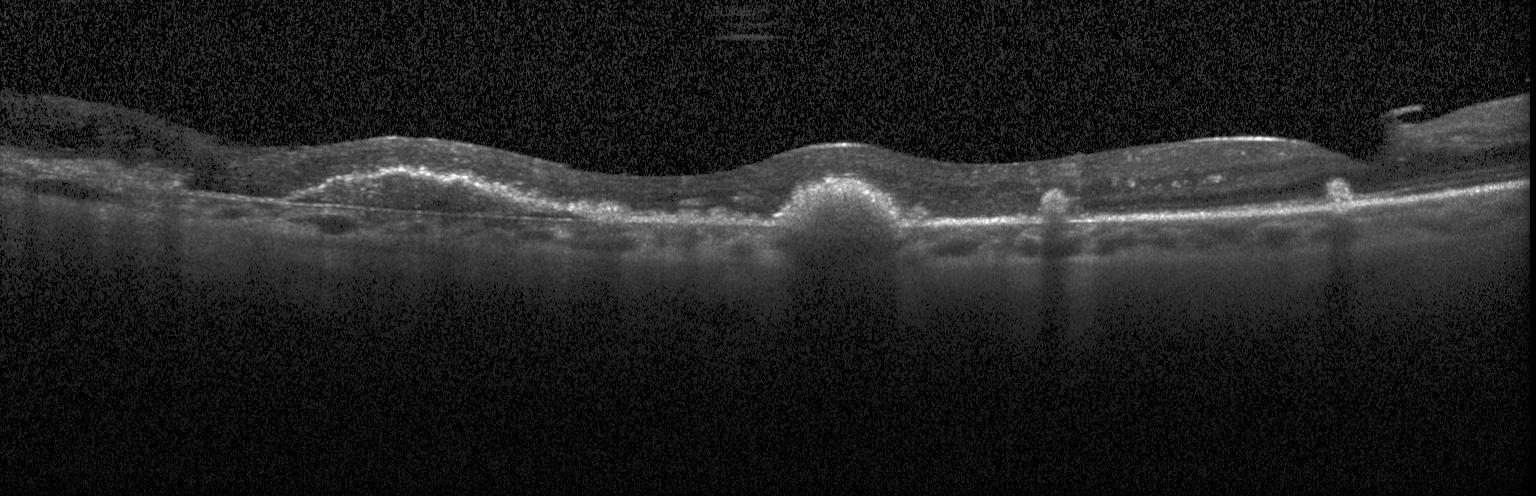 Spectral-domain optical coherence tomography. Macular scan. Heidelberg Spectralis OCT system. Retinal OCT cross-section
Impression: a choroidal neovascular membrane.